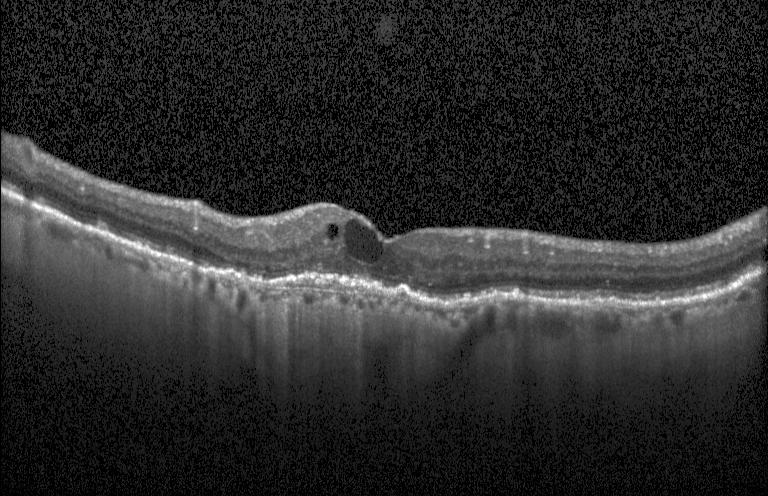

SD-OCT; acquired on a Heidelberg Spectralis; through the macula; OCT B-scan
A choroidal neovascular membrane.